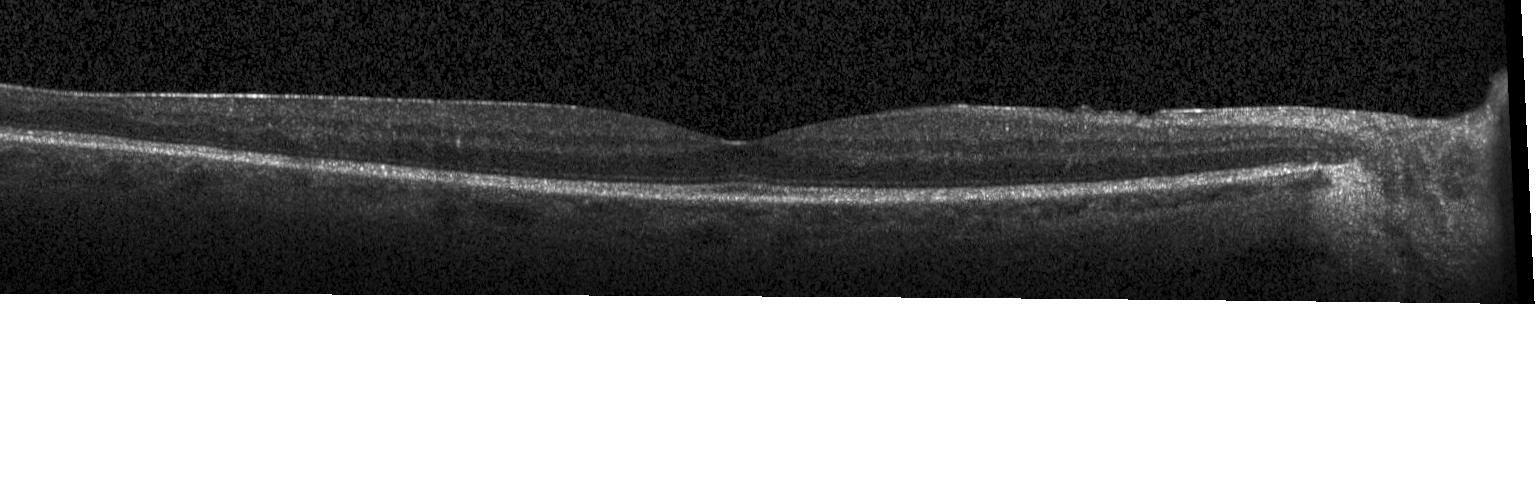
Fovea-centered, spectral-domain OCT, retinal OCT cross-section — Diagnosis: neither choroidal neovascularization, diabetic macular edema, nor drusen.